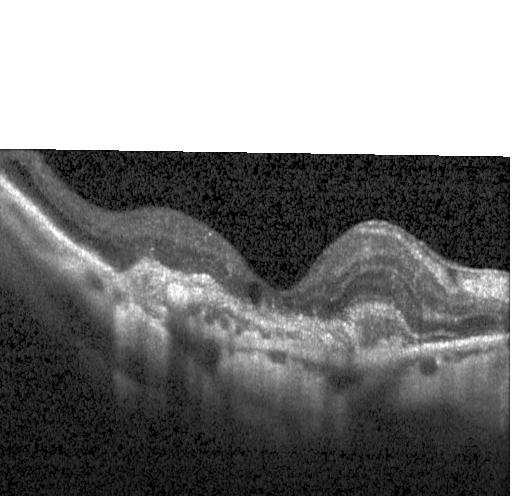 OCT finding: choroidal neovascularization (CNV).